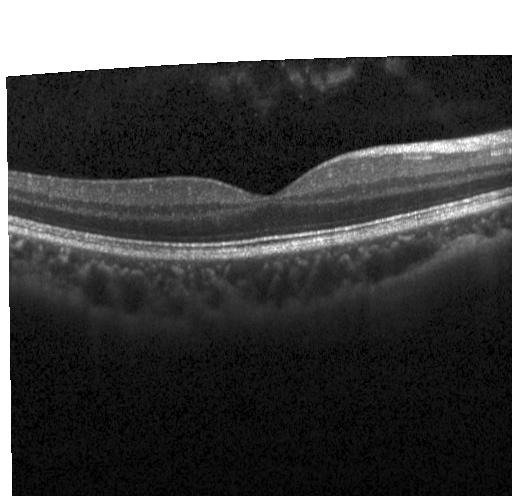 Optical coherence tomography B-scan, spectral-domain OCT — Assessment: no evidence of CNV, DME, or drusen.